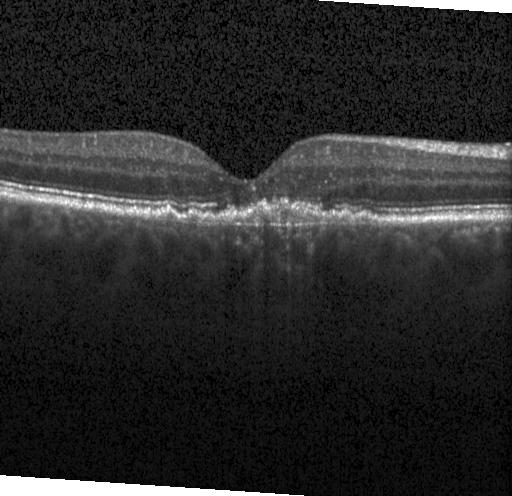 Spectral-domain OCT B-scan: choroidal neovascularization.